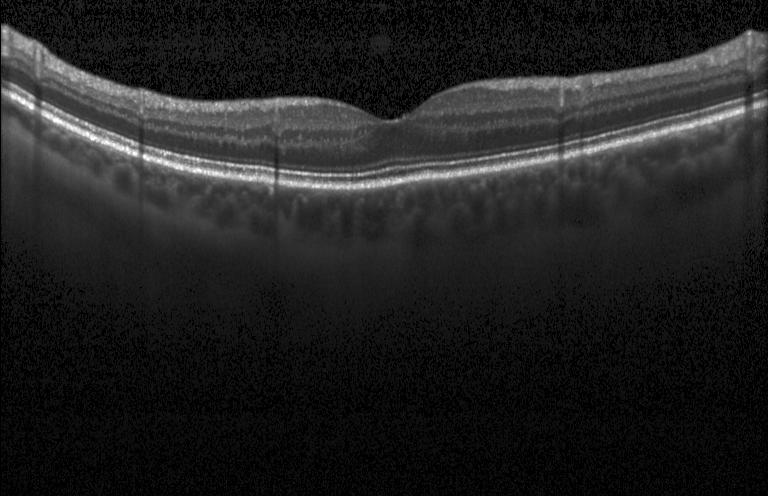 Optical coherence tomography scan. Centered on the fovea. SD-OCT — Assessment: no CNV, DME, or drusen.